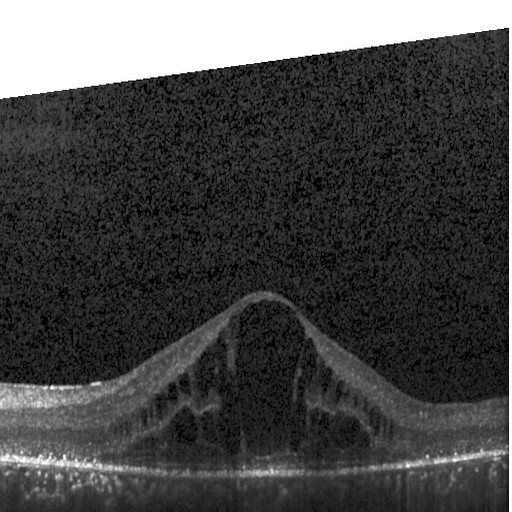
The scan shows diabetic macular edema.